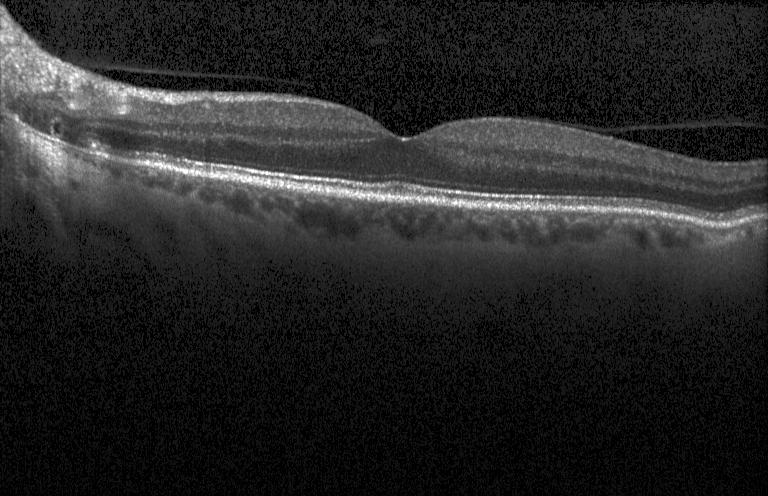

Optical coherence tomography B-scan. Horizontal scan through the fovea. Heidelberg Spectralis OCT system. Spectral-domain optical coherence tomography.
OCT finding: no choroidal neovascularization, no diabetic macular edema, and no drusen.